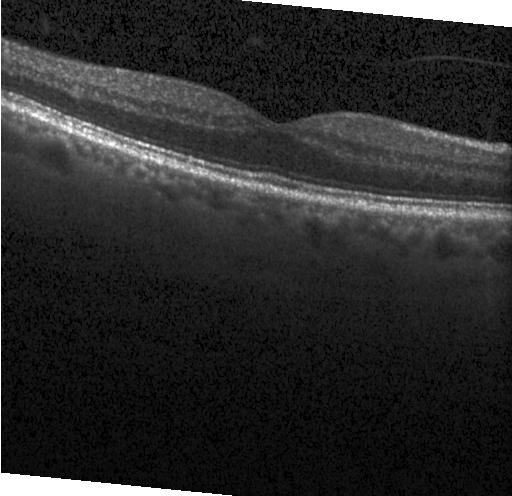
OCT B-scan. Diagnosis: no evidence of choroidal neovascularization, diabetic macular edema, or drusen.